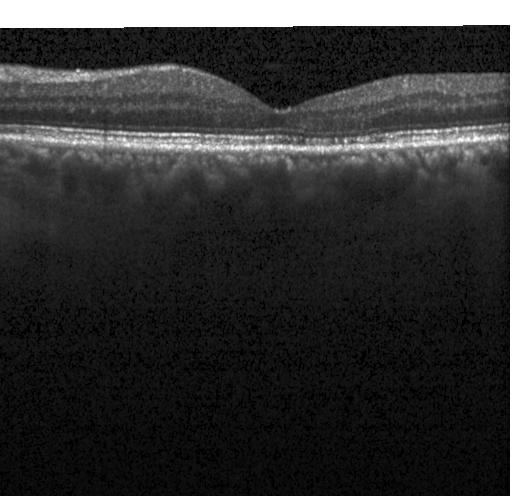 Diagnosis: no choroidal neovascularization, no diabetic macular edema, and no drusen.